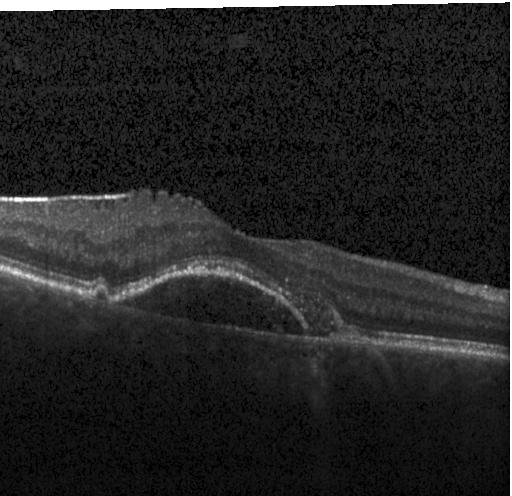 Heidelberg Spectralis OCT system · retinal OCT cross-section. Finding: choroidal neovascularization (CNV).